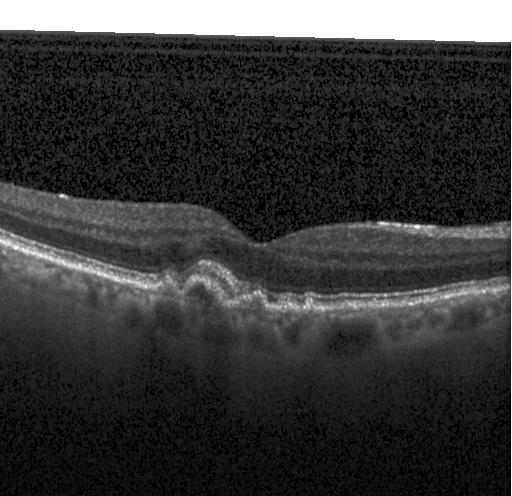

CNV.